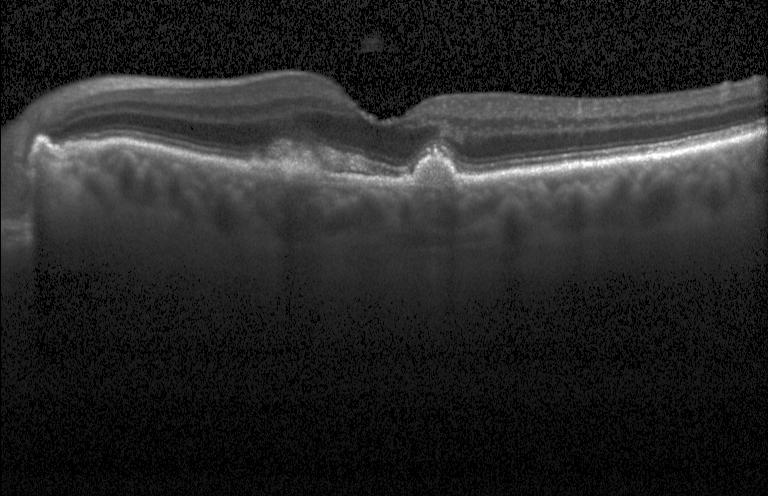

Impression: CNV.